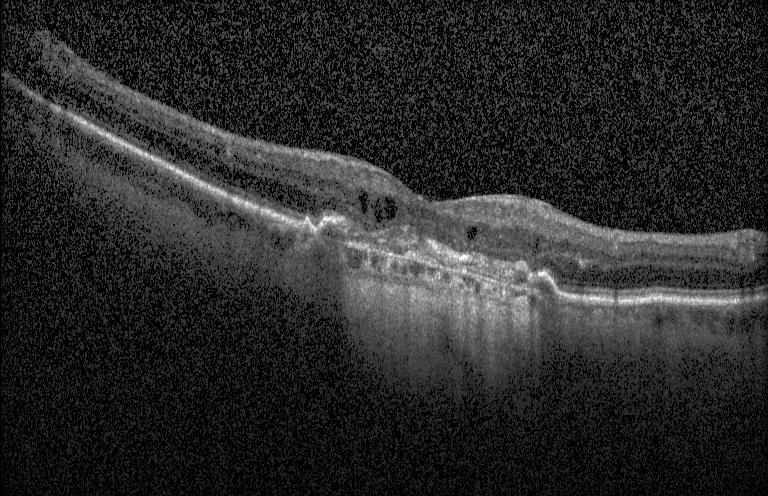 SD-OCT. Retinal OCT B-scan. Diagnosis: CNV.